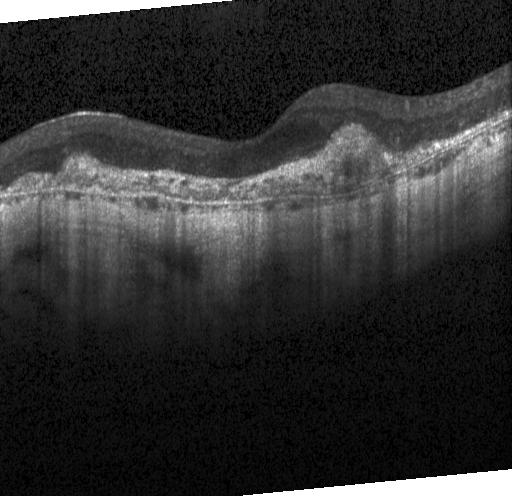 Macular scan · optical coherence tomography scan · spectral-domain OCT. Impression: choroidal neovascularization (CNV).